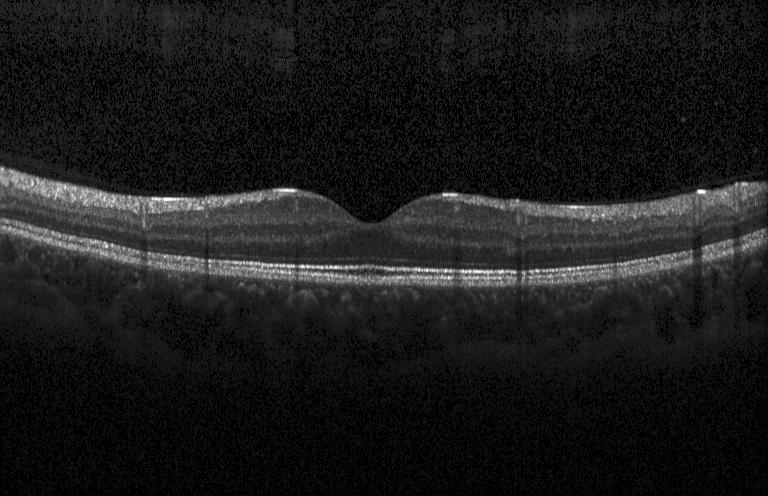
Retinal OCT cross-section. Diagnosis: neither choroidal neovascularization, diabetic macular edema, nor drusen.